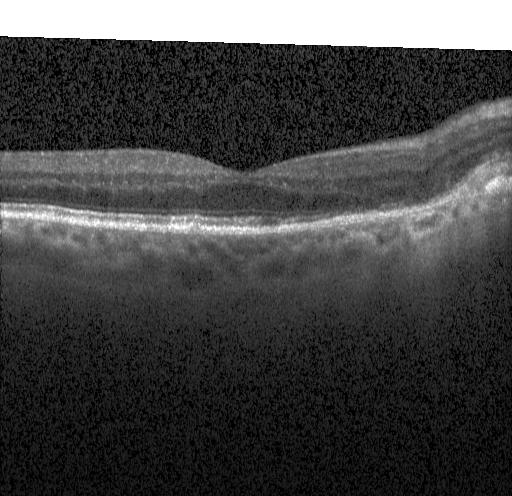 Macular OCT demonstrating a choroidal neovascular membrane.